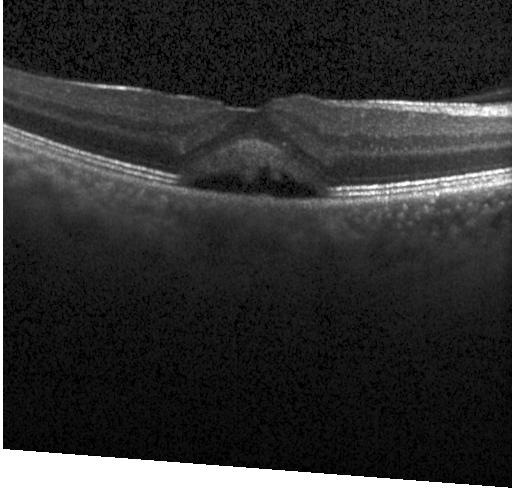

Retinal OCT cross-section showing a choroidal neovascular membrane.